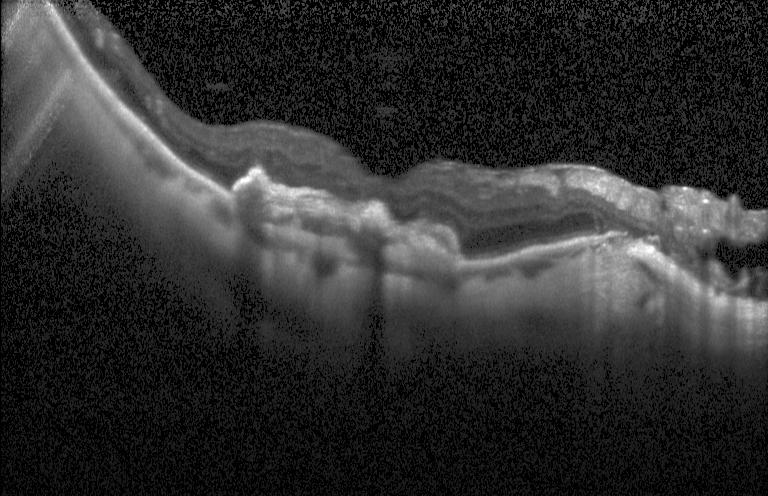
Optical coherence tomography scan
Diagnosis: a choroidal neovascular membrane.